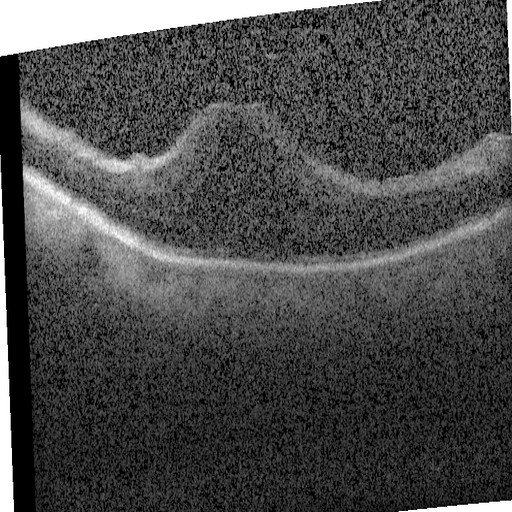

SD-OCT; fovea-centered; retinal OCT B-scan; acquired on a Heidelberg Spectralis.
Finding: diabetic macular edema.